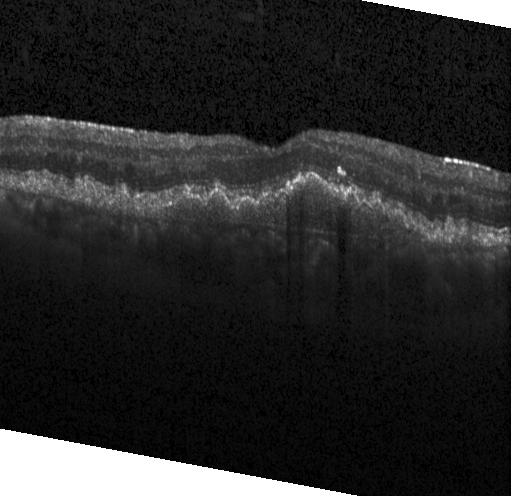 Finding: choroidal neovascularization.